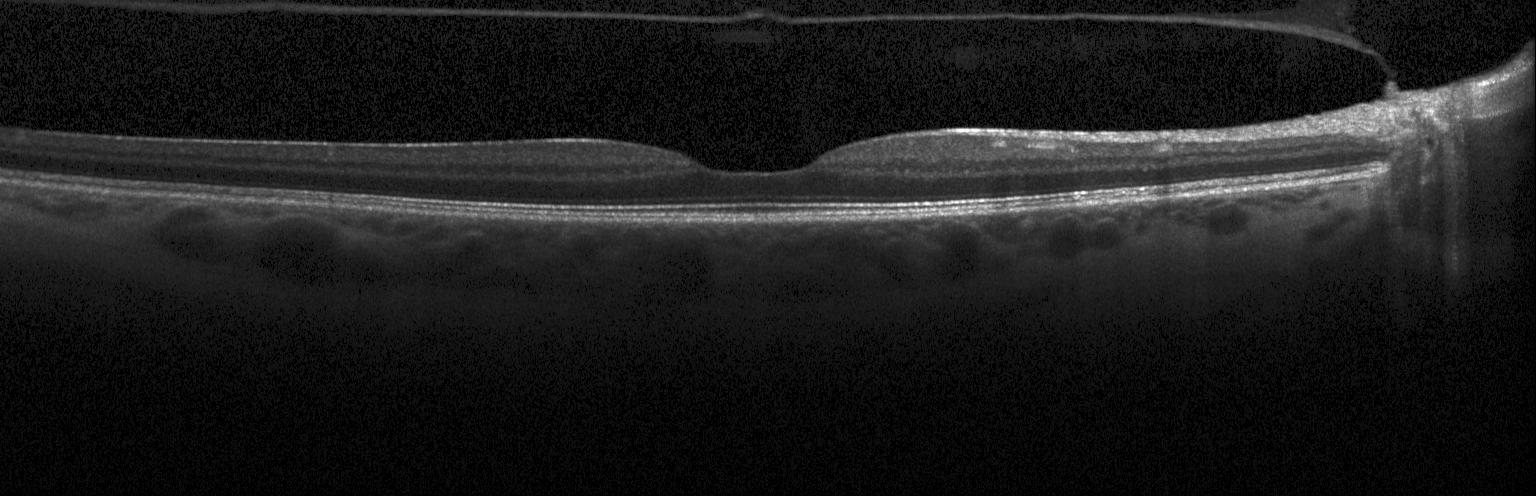
Assessment: neither choroidal neovascularization, diabetic macular edema, nor drusen.